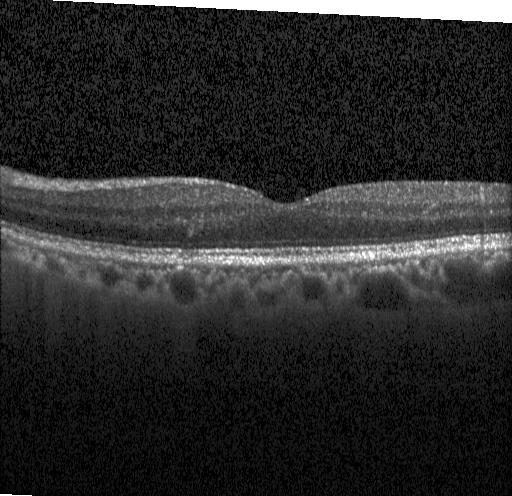
Optical coherence tomography B-scan — No choroidal neovascularization, no diabetic macular edema, and no drusen.